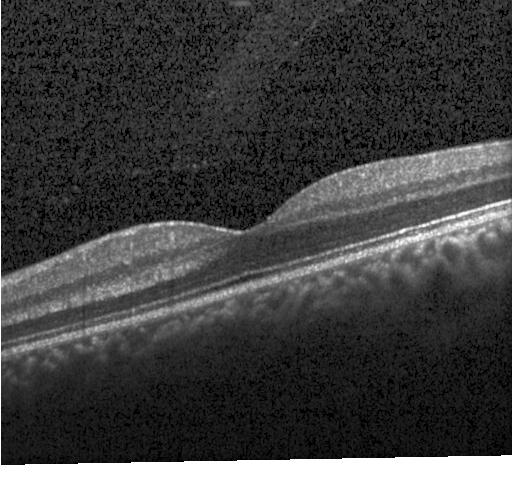

Optical coherence tomography scan · Heidelberg Spectralis · spectral-domain optical coherence tomography. Macular OCT: no choroidal neovascularization, no diabetic macular edema, and no drusen.